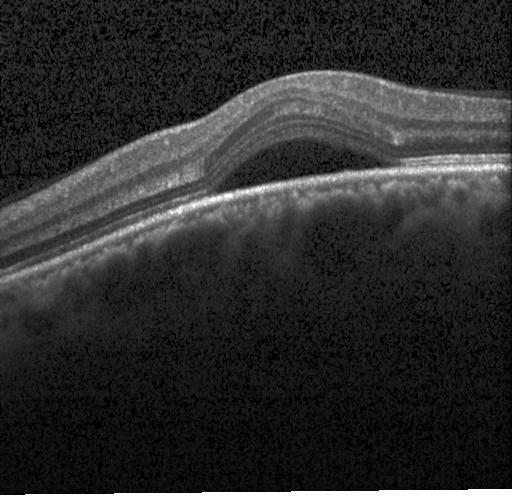 OCT finding: choroidal neovascularization (CNV).